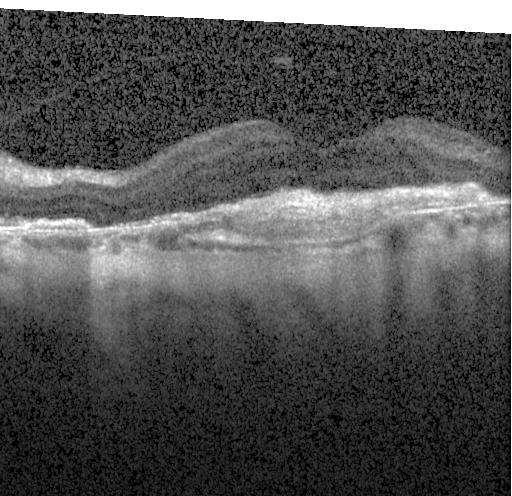 Optical coherence tomography scan; spectral-domain optical coherence tomography; Heidelberg Spectralis. Impression: a choroidal neovascular membrane.